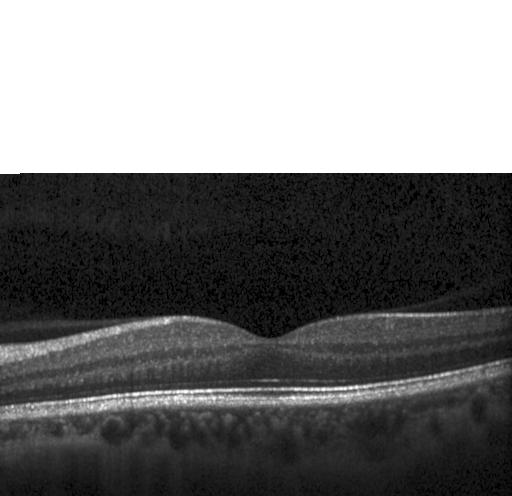 OCT finding: no choroidal neovascularization, diabetic macular edema, or drusen.